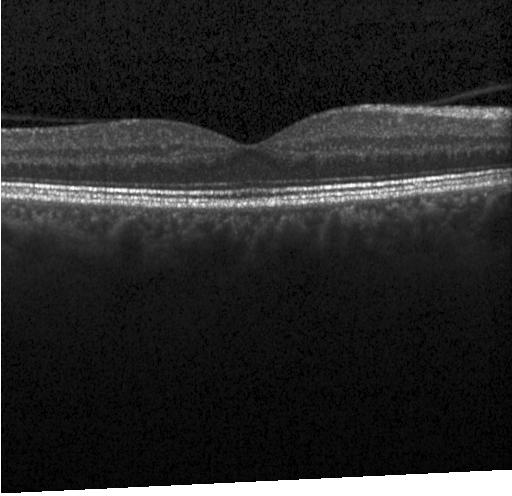

Retinal OCT B-scan — Dx: no evidence of CNV, DME, or drusen.